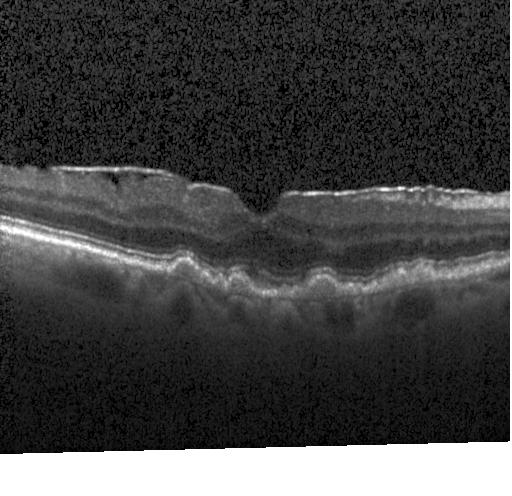
Finding: drusen.